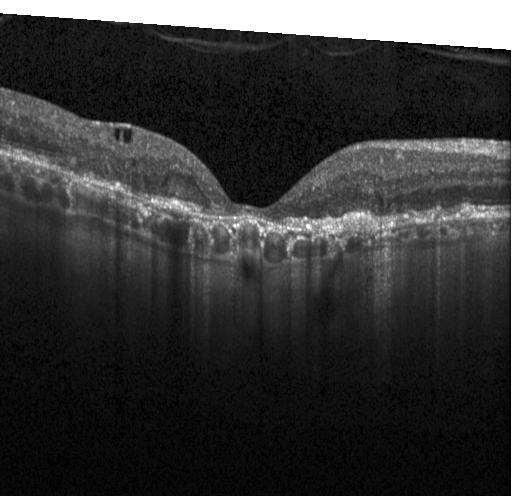
Through the macula · spectral-domain OCT · OCT B-scan · acquired on a Heidelberg Spectralis. Assessment: choroidal neovascularization.